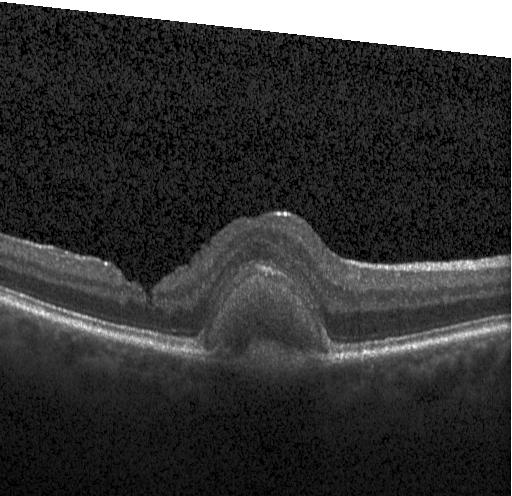

Acquired on a Heidelberg Spectralis · spectral-domain OCT · optical coherence tomography scan · fovea-centered
Macular OCT: a choroidal neovascular membrane.